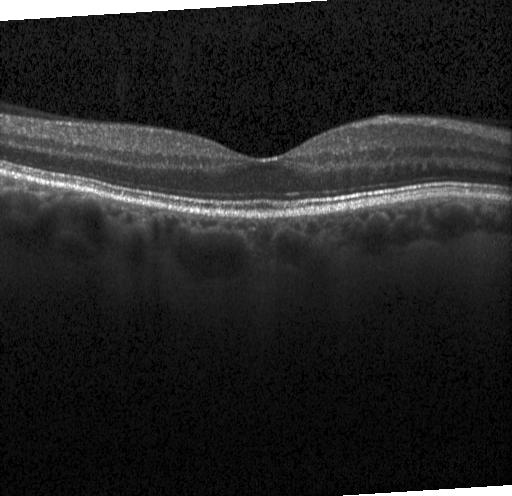 Fovea-centered · spectral-domain OCT · Heidelberg Spectralis · optical coherence tomography B-scan — This B-scan demonstrates no evidence of CNV, DME, or drusen.